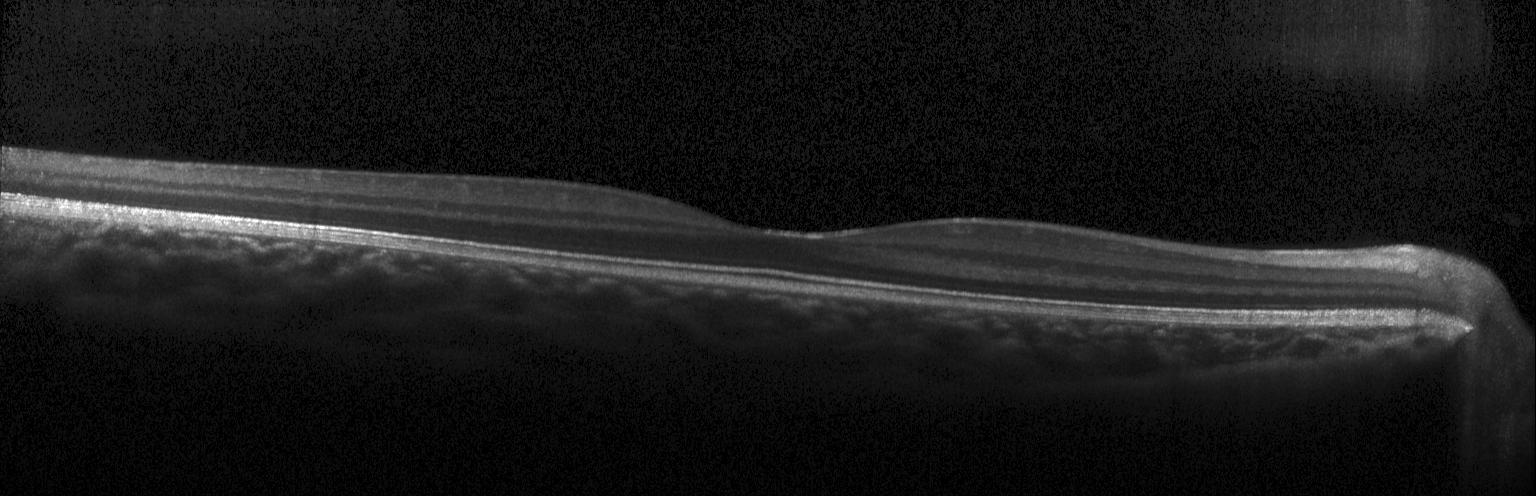

Optical coherence tomography scan · centered on the fovea. This B-scan demonstrates no choroidal neovascularization, diabetic macular edema, or drusen.